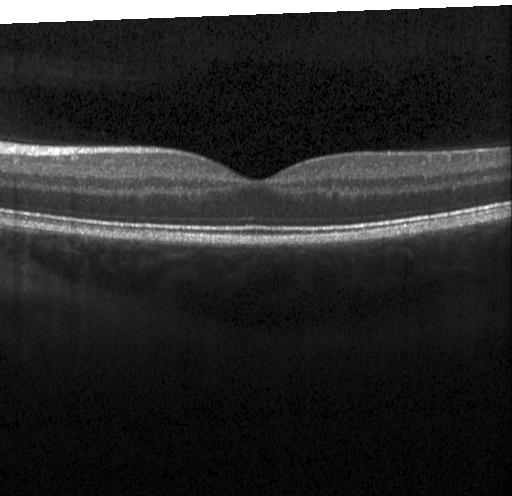

The scan shows neither CNV, DME, nor drusen.